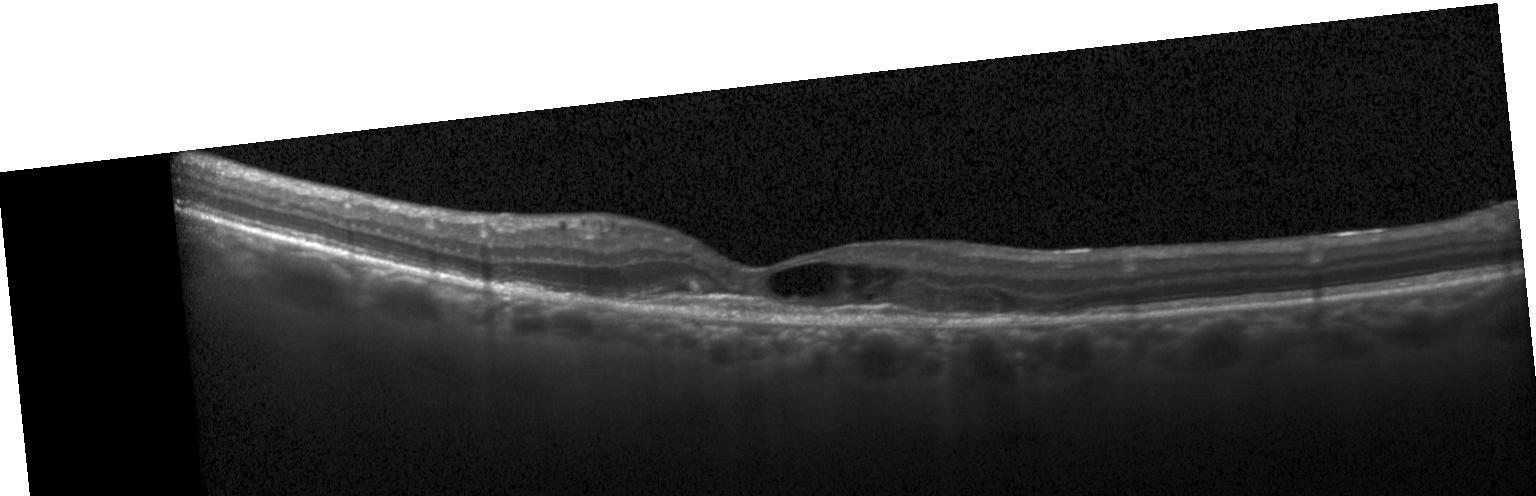 OCT B-scan.
Finding: CNV.